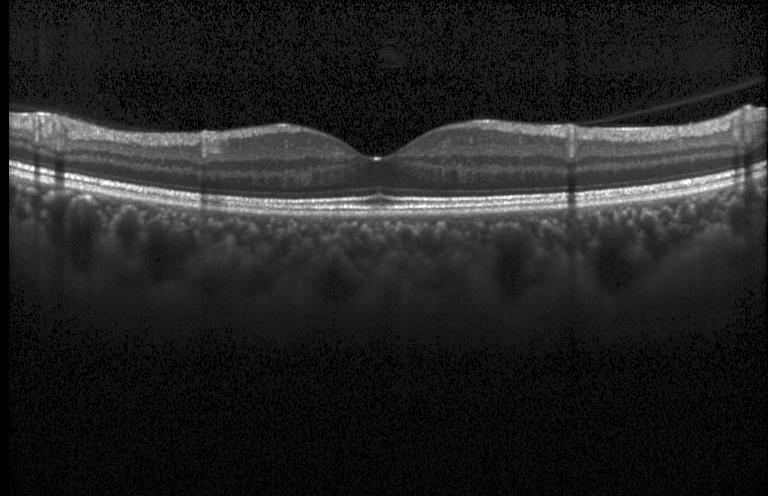

Macular OCT demonstrating no evidence of CNV, DME, or drusen.